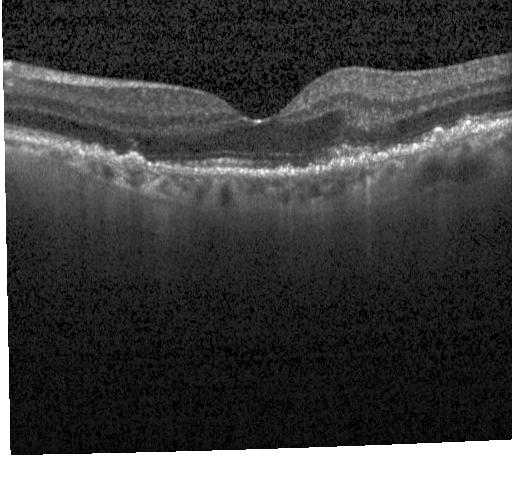

Fovea-centered. Instrument: Heidelberg Spectralis. SD-OCT. Retinal OCT cross-section.
Dx: multiple drusen.